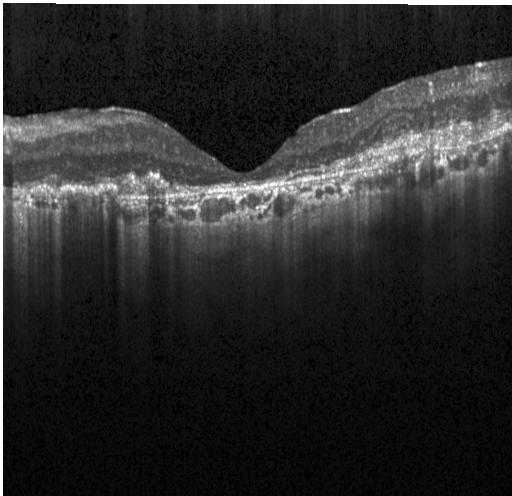 OCT B-scan · horizontal scan through the fovea · instrument: Heidelberg Spectralis. Impression: choroidal neovascularization.